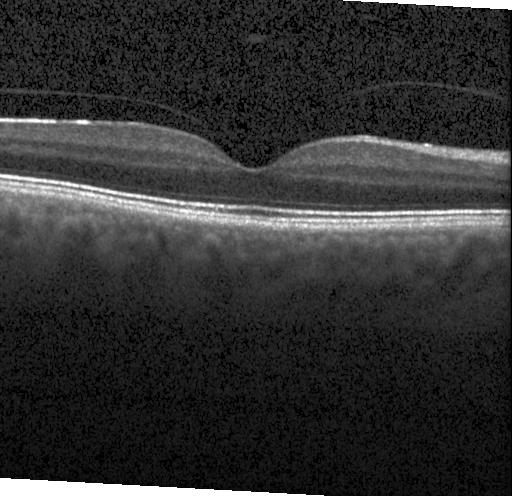
Horizontal scan through the fovea · retinal OCT B-scan
No evidence of choroidal neovascularization, diabetic macular edema, or drusen.